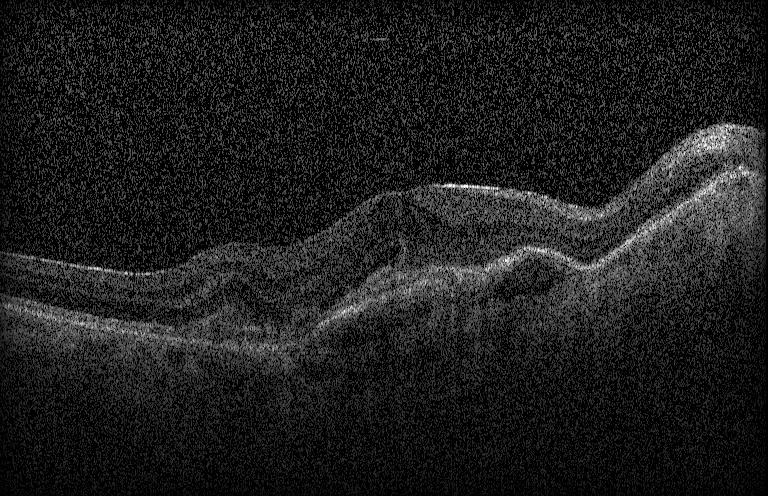
Retinal OCT B-scan; Heidelberg Spectralis; SD-OCT; macular scan
Diagnosis: a choroidal neovascular membrane.